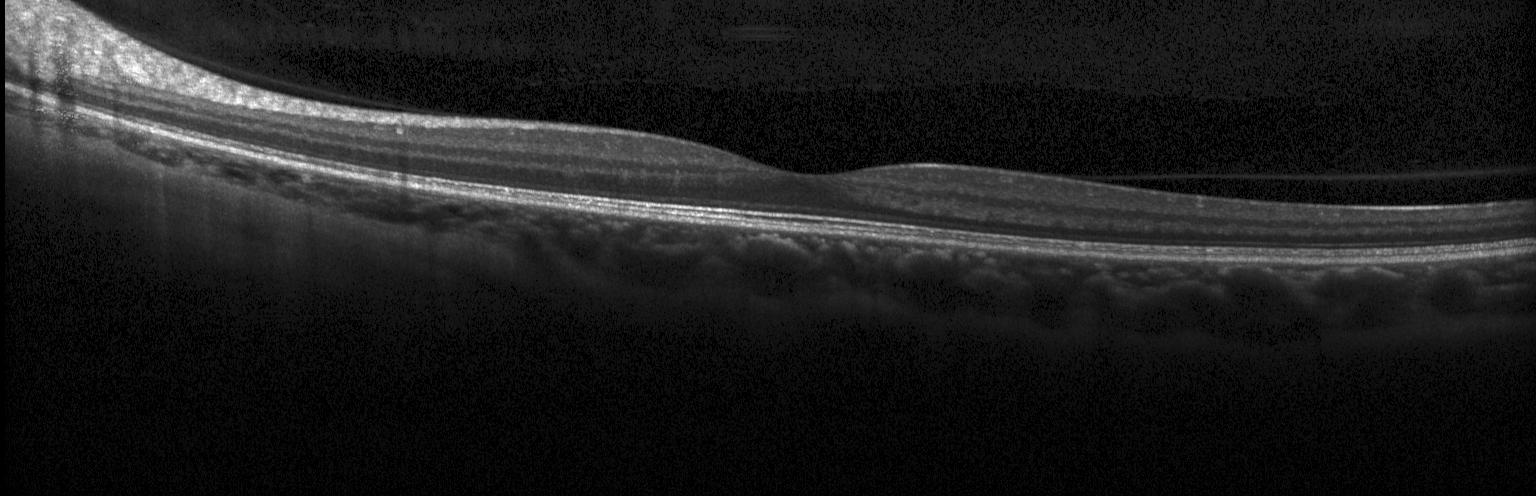 Diagnosis: no evidence of choroidal neovascularization, diabetic macular edema, or drusen.